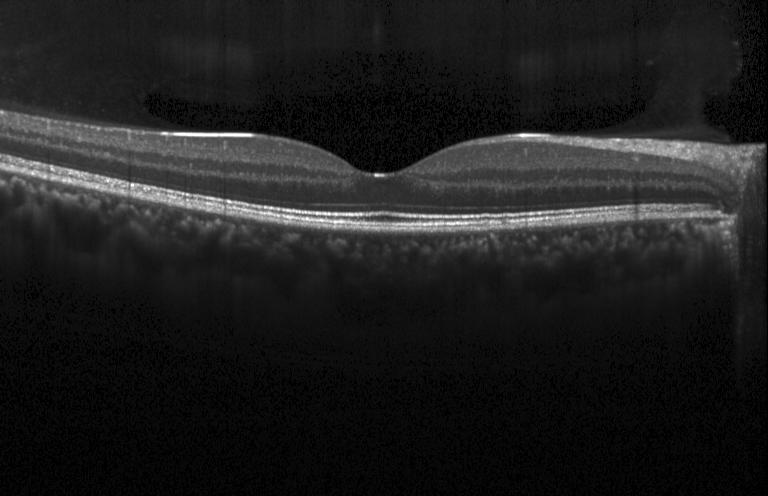

Spectral-domain OCT · acquired on a Heidelberg Spectralis · optical coherence tomography B-scan · through the macula
Macular OCT: no evidence of CNV, DME, or drusen.